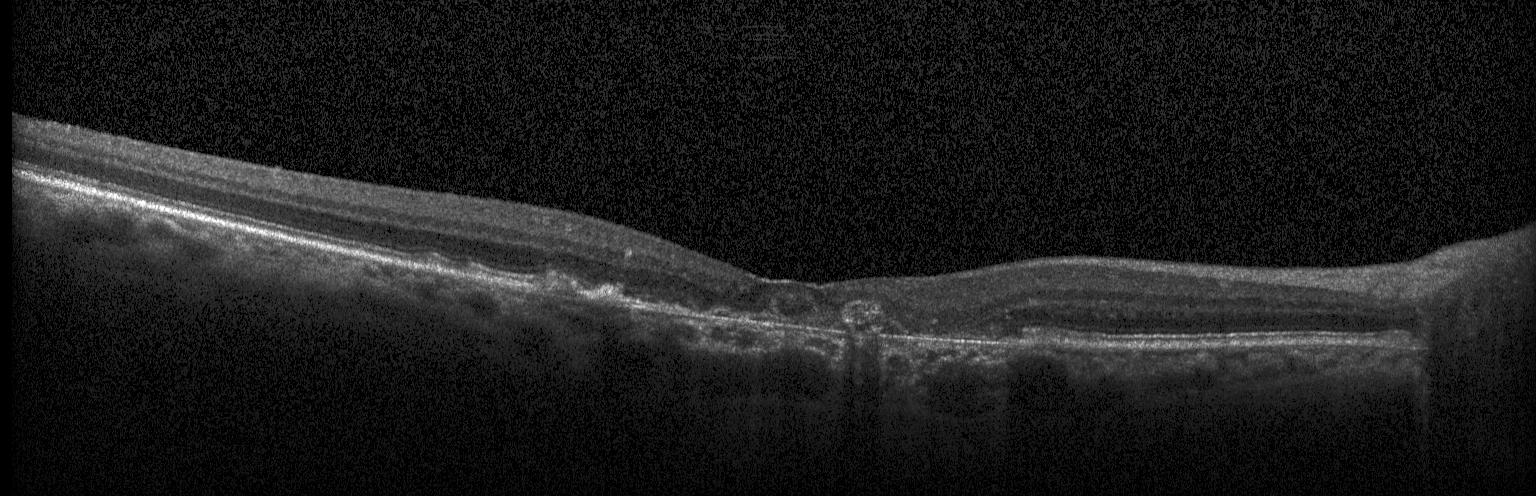

Spectral-domain OCT; OCT B-scan; through the macula; Heidelberg Spectralis OCT system. Impression: a choroidal neovascular membrane.